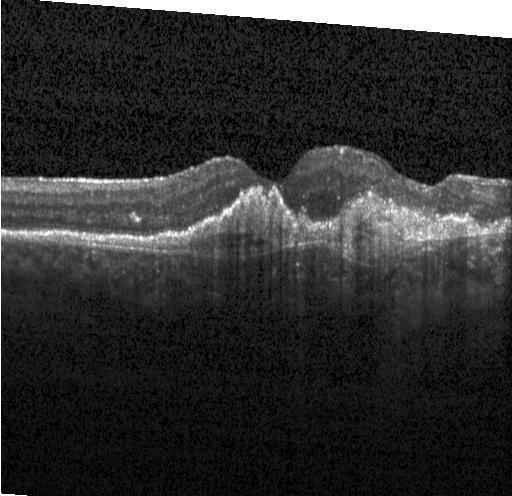 SD-OCT. Heidelberg Spectralis. Horizontal scan through the fovea. Optical coherence tomography B-scan — This B-scan demonstrates a choroidal neovascular membrane.